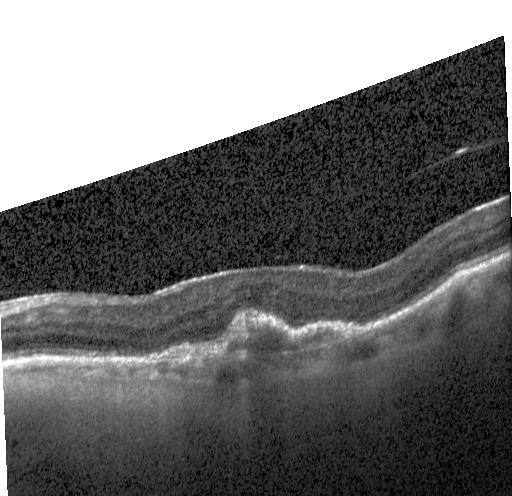
Assessment: choroidal neovascularization.